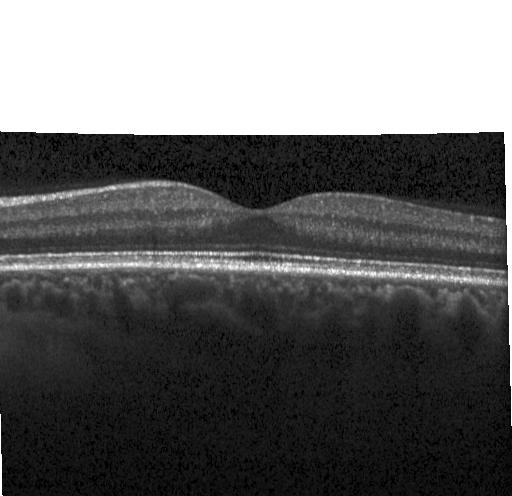

Macular OCT demonstrating no choroidal neovascularization, diabetic macular edema, or drusen.